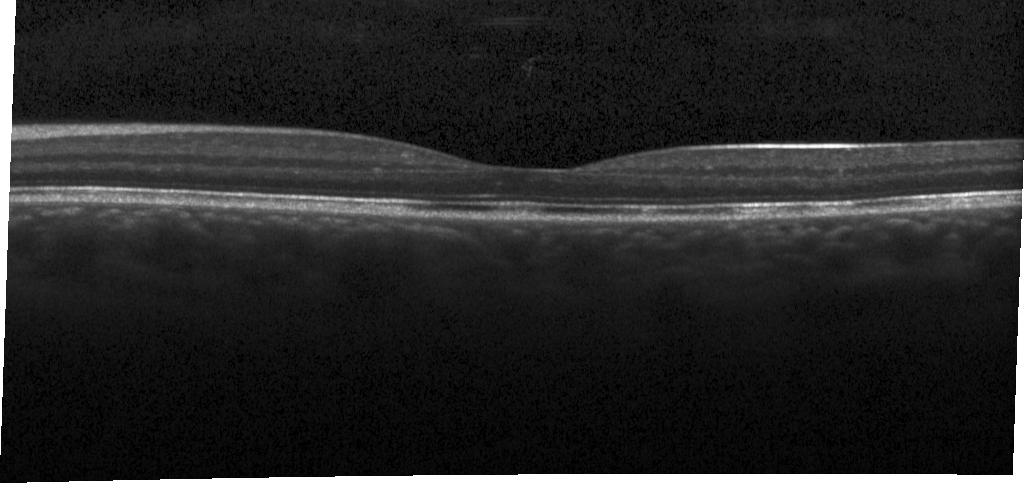 SD-OCT. OCT B-scan
Dx: no choroidal neovascularization, diabetic macular edema, or drusen.